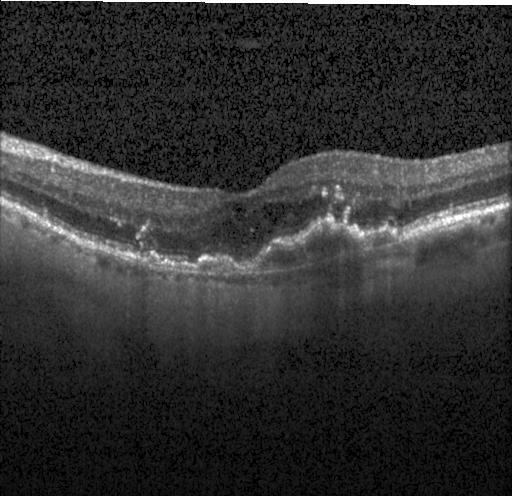

Centered on the fovea. Optical coherence tomography scan.
Choroidal neovascularization.